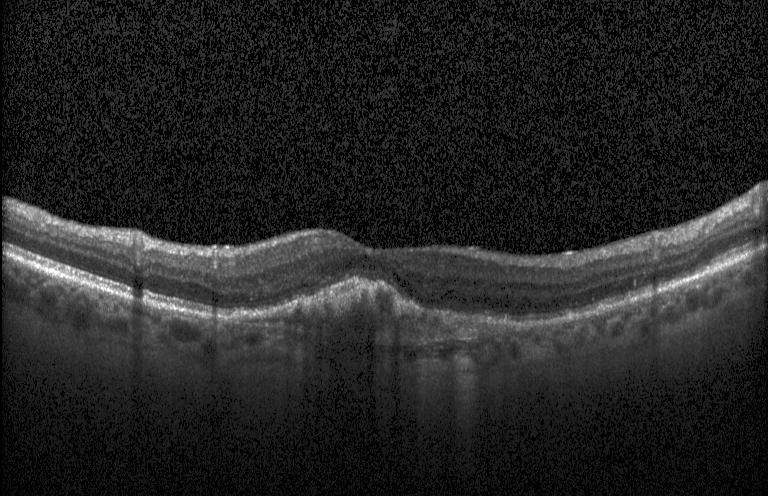

SD-OCT. OCT B-scan. Assessment: a choroidal neovascular membrane.